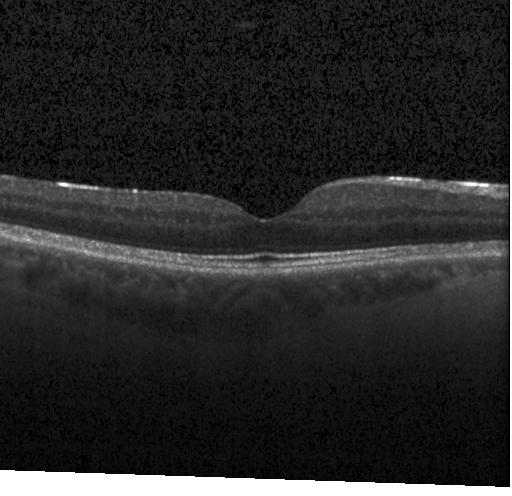 Spectral-domain OCT B-scan: no evidence of CNV, DME, or drusen.